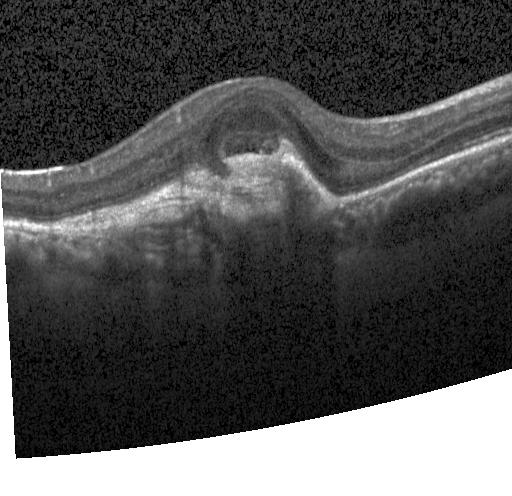

Centered on the fovea, spectral-domain OCT, optical coherence tomography B-scan — Dx: a choroidal neovascular membrane.